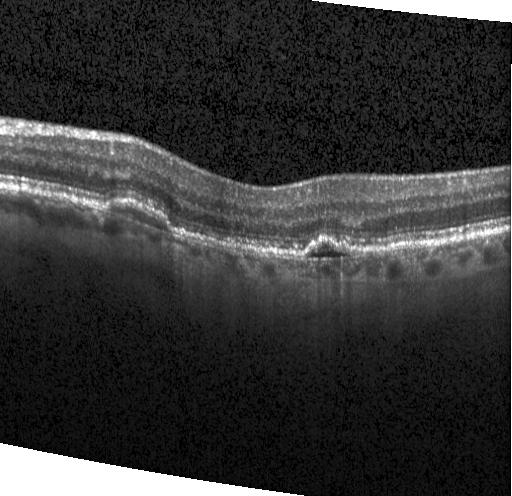

Retinal OCT cross-section; Heidelberg Spectralis OCT system; spectral-domain OCT; centered on the fovea. Choroidal neovascularization.